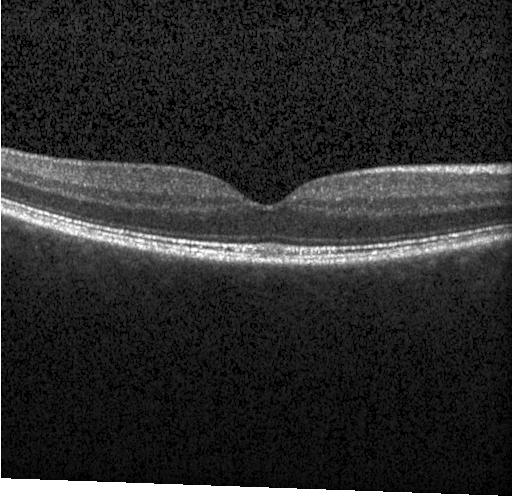 OCT B-scan showing no choroidal neovascularization, no diabetic macular edema, and no drusen.